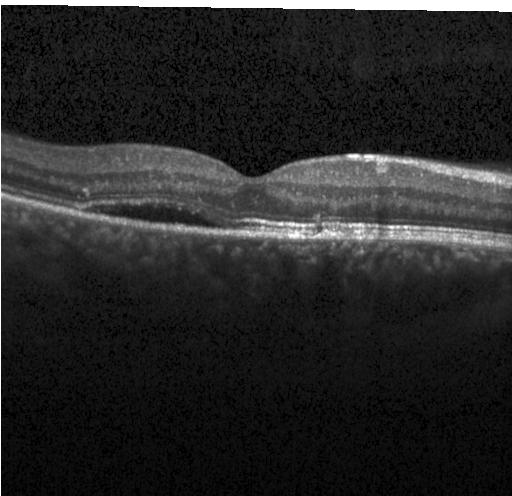

OCT line scan, macular scan
Diagnosis: choroidal neovascularization.